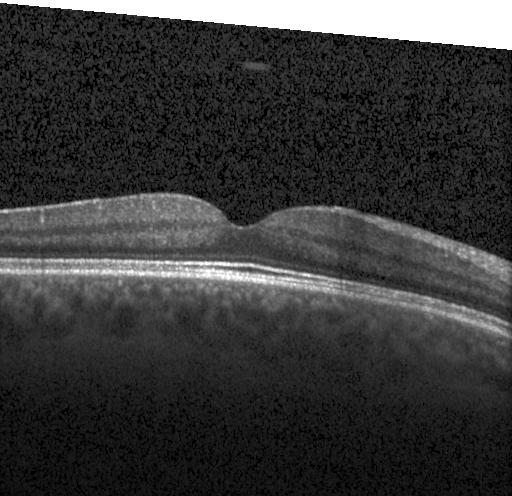

OCT B-scan showing no choroidal neovascularization, no diabetic macular edema, and no drusen.